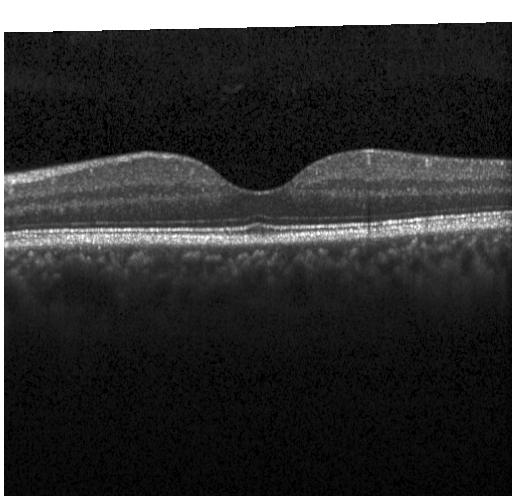 Fovea-centered. Retinal OCT B-scan. SD-OCT.
No choroidal neovascularization, no diabetic macular edema, and no drusen.